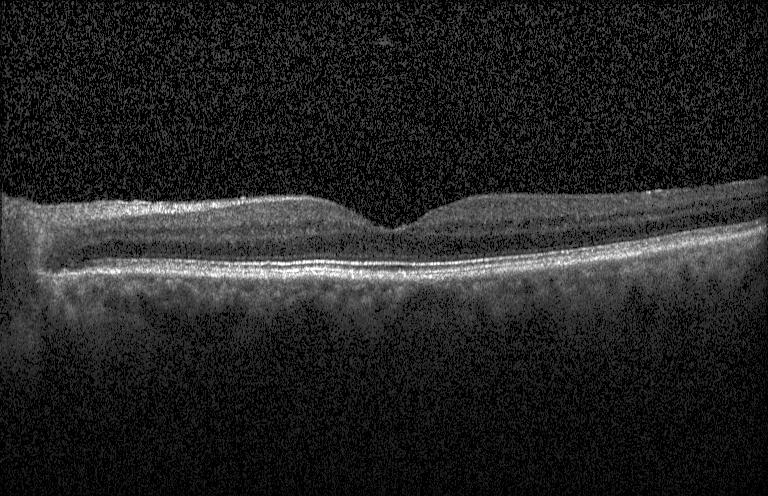

Macular scan; OCT line scan; Heidelberg Spectralis
Macular OCT: no choroidal neovascularization, diabetic macular edema, or drusen.